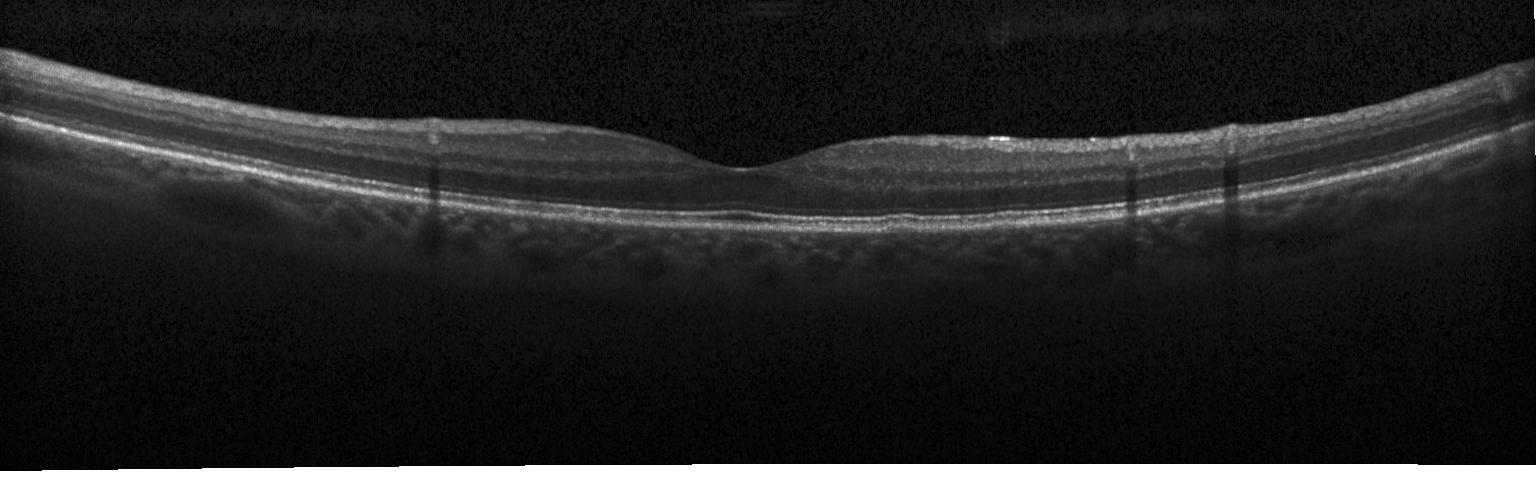 Horizontal scan through the fovea, acquired on a Heidelberg Spectralis, retinal OCT B-scan, spectral-domain optical coherence tomography.
No choroidal neovascularization, no diabetic macular edema, and no drusen.